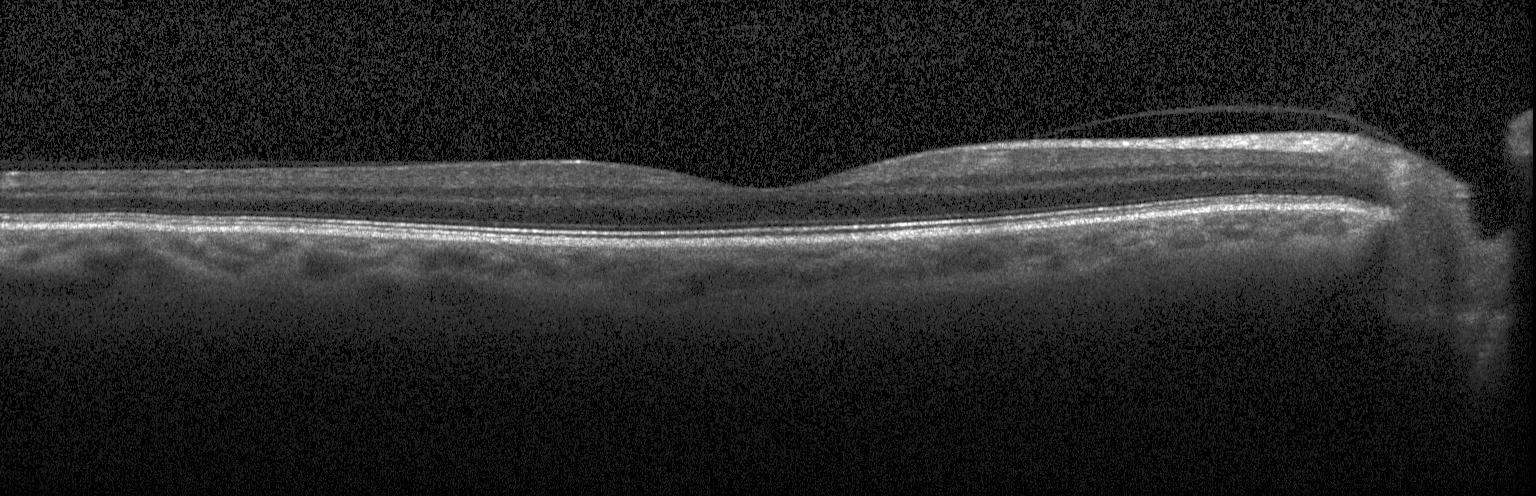 Optical coherence tomography B-scan, SD-OCT — Diagnosis: no evidence of choroidal neovascularization, diabetic macular edema, or drusen.